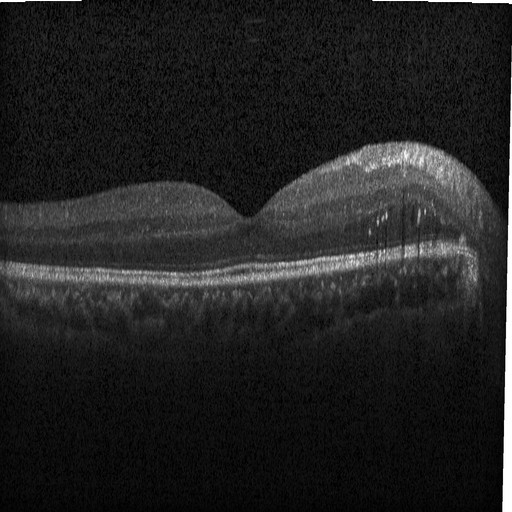 Macular OCT: diabetic macular edema.